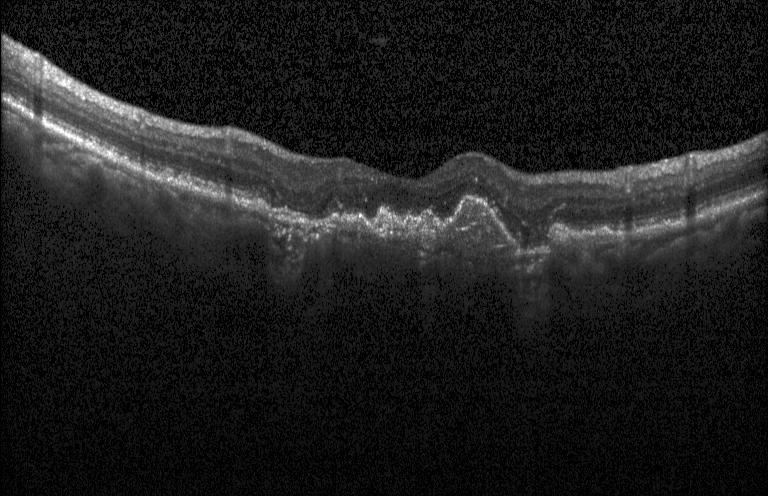

Dx: a choroidal neovascular membrane.